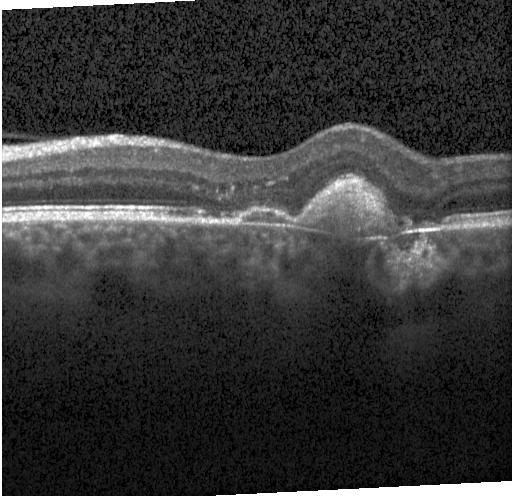

This B-scan demonstrates choroidal neovascularization (CNV).